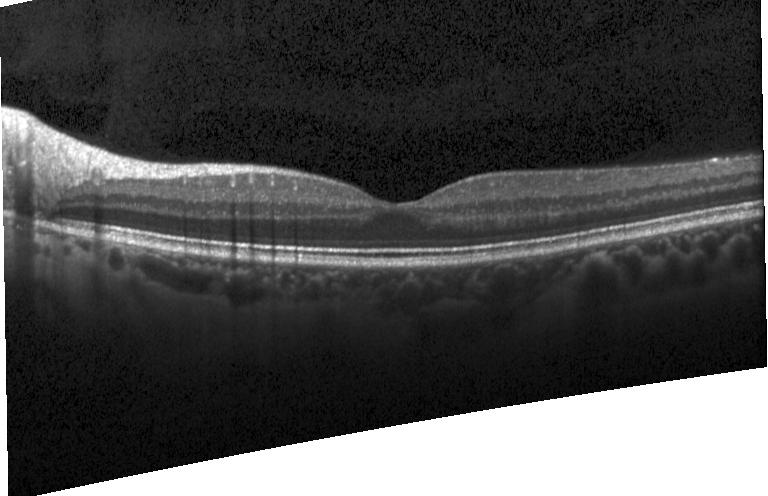

Spectral-domain OCT · retinal OCT cross-section.
Impression: no evidence of CNV, DME, or drusen.